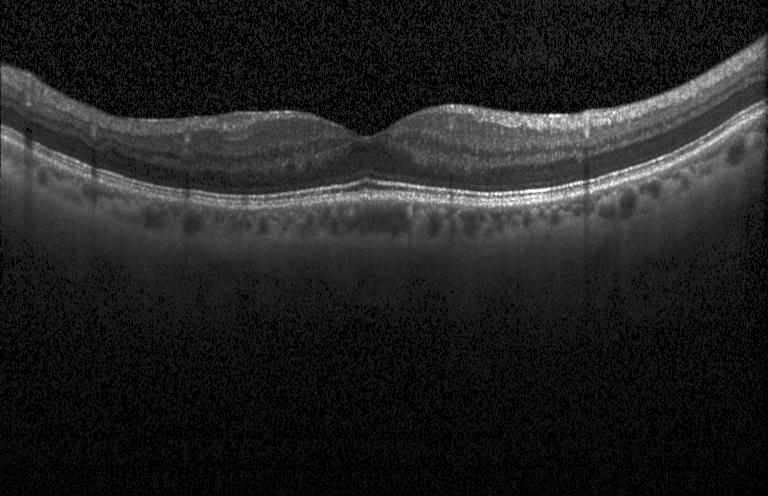

SD-OCT · OCT B-scan. Finding: no choroidal neovascularization, no diabetic macular edema, and no drusen.